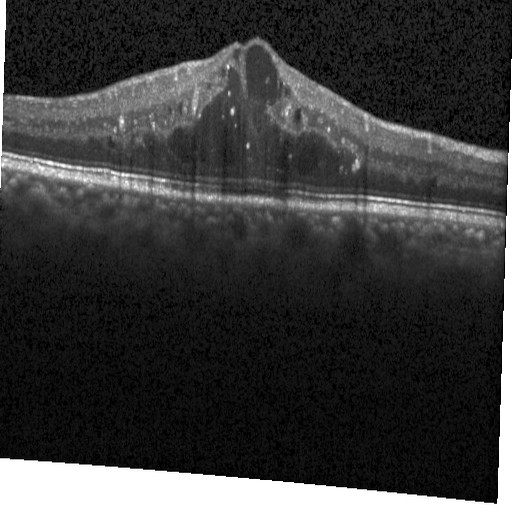 Spectral-domain OCT, Heidelberg Spectralis, optical coherence tomography B-scan, through the macula. Finding: diabetic macular edema.